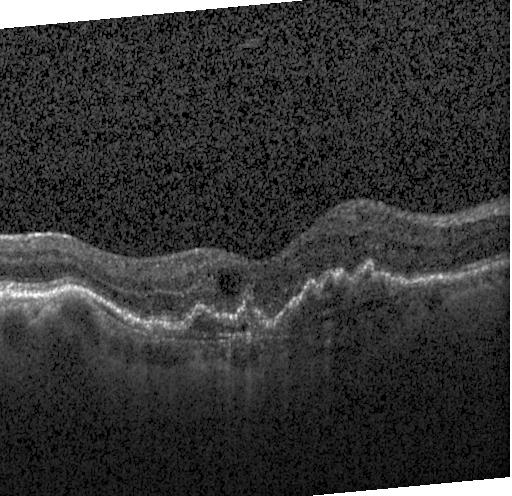

Spectral-domain OCT · OCT B-scan · acquired on a Heidelberg Spectralis
Diagnosis: choroidal neovascularization.